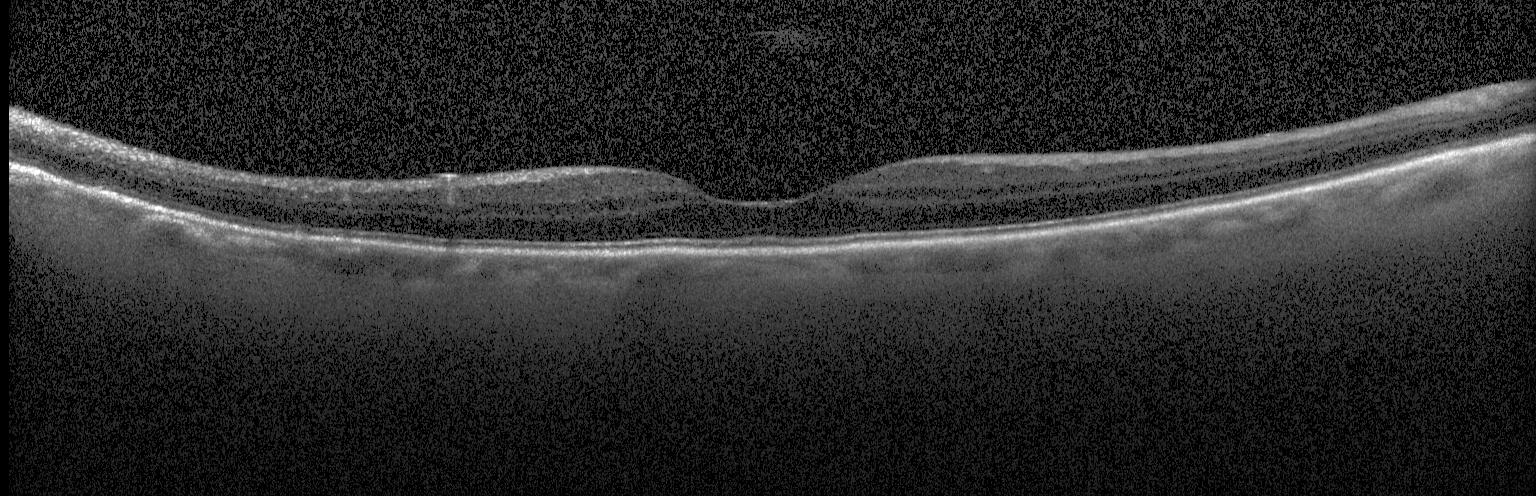 This B-scan demonstrates no evidence of choroidal neovascularization, diabetic macular edema, or drusen.